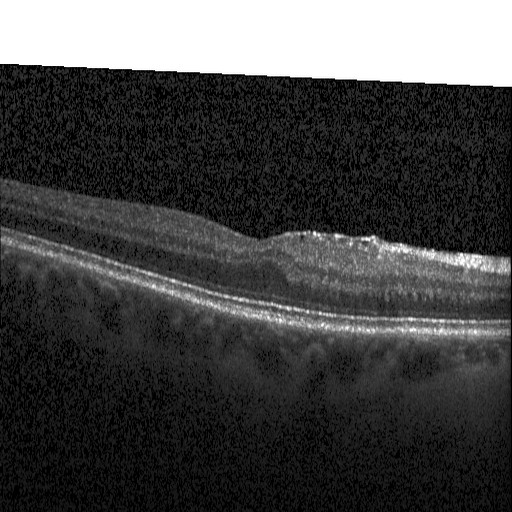

Diagnosis: diabetic macular edema (DME).